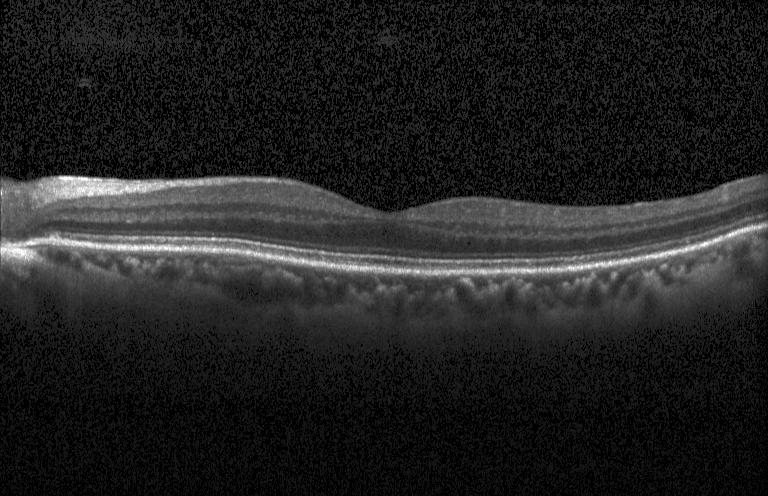
OCT finding: no CNV, DME, or drusen.